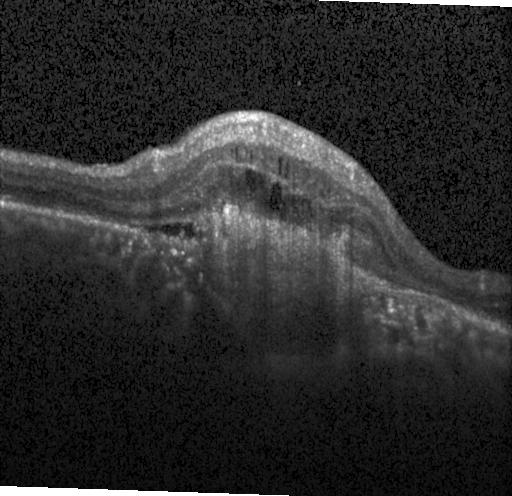
The scan shows choroidal neovascularization.